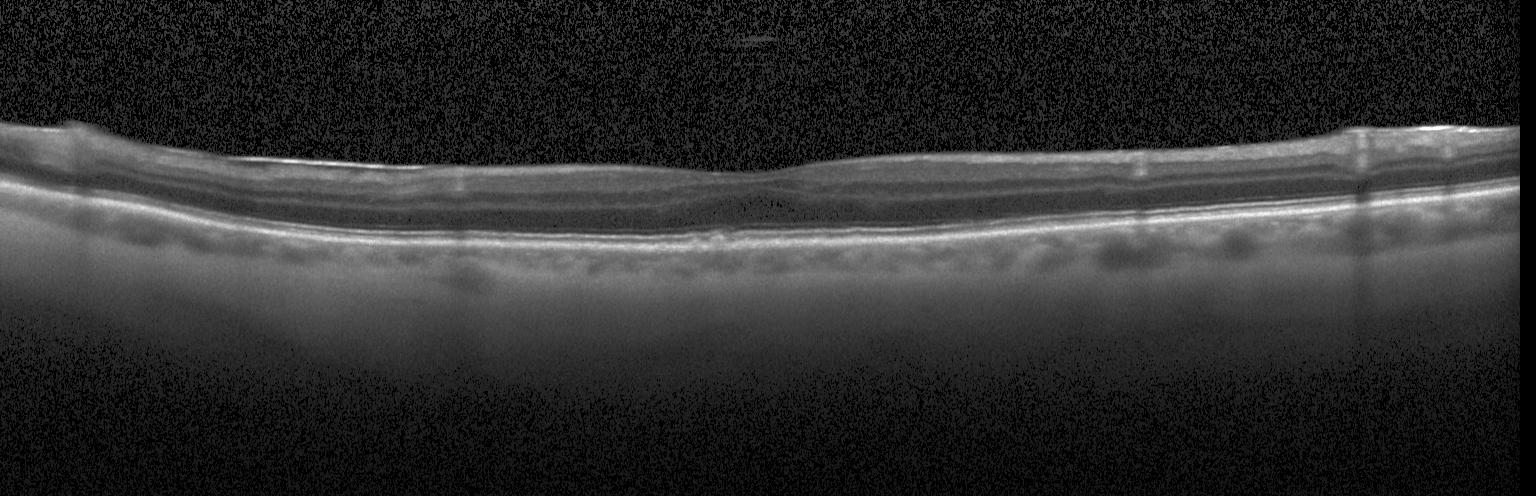

Diagnosis: sub-RPE drusenoid deposits.